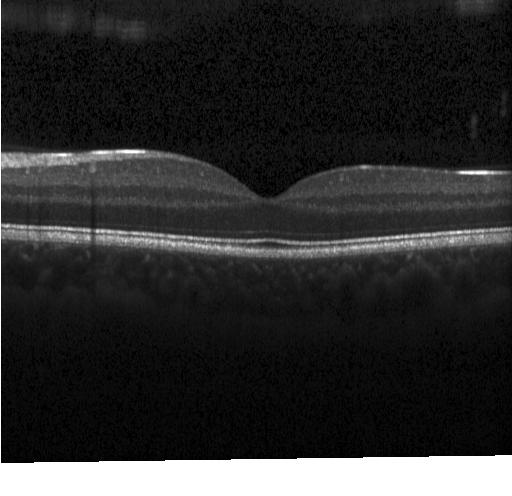 Centered on the fovea. OCT line scan. SD-OCT.
Assessment: no choroidal neovascularization, diabetic macular edema, or drusen.